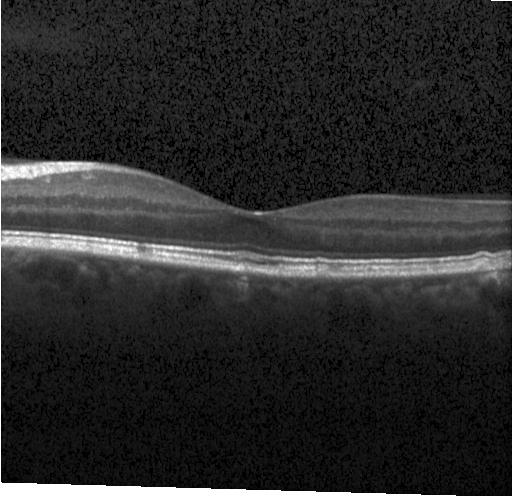
The scan shows sub-RPE drusenoid deposits.